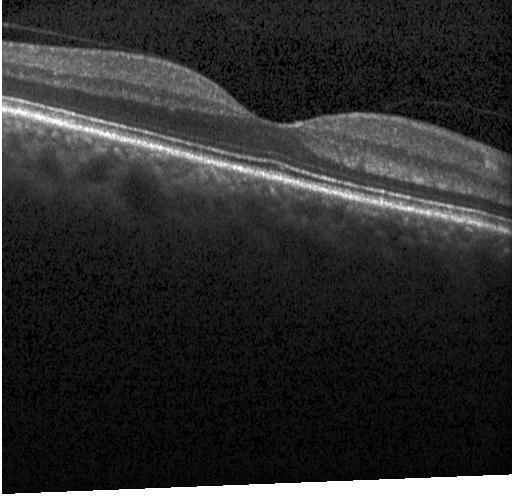

Optical coherence tomography scan
Impression: no evidence of CNV, DME, or drusen.